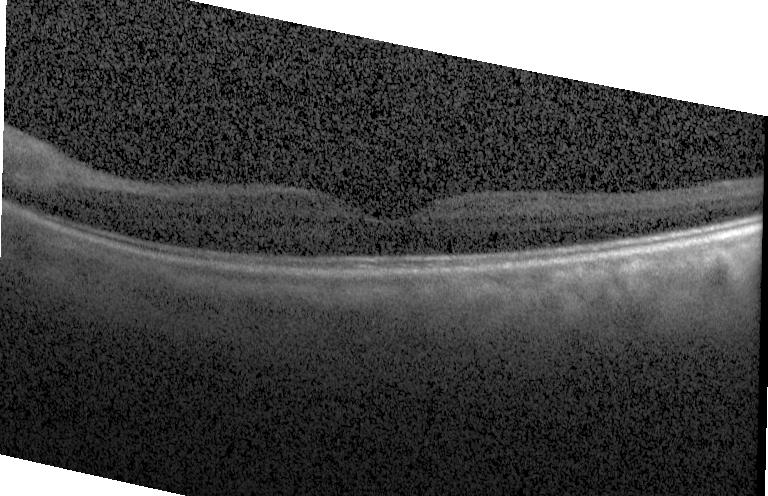
SD-OCT; acquired on a Heidelberg Spectralis; fovea-centered; retinal OCT cross-section — No choroidal neovascularization, no diabetic macular edema, and no drusen.